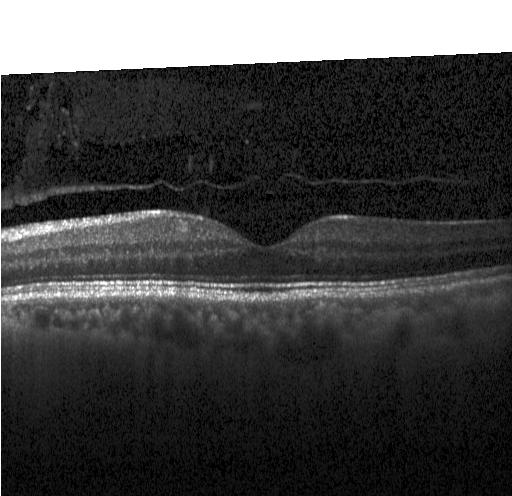

Optical coherence tomography B-scan.
Finding: no choroidal neovascularization, no diabetic macular edema, and no drusen.